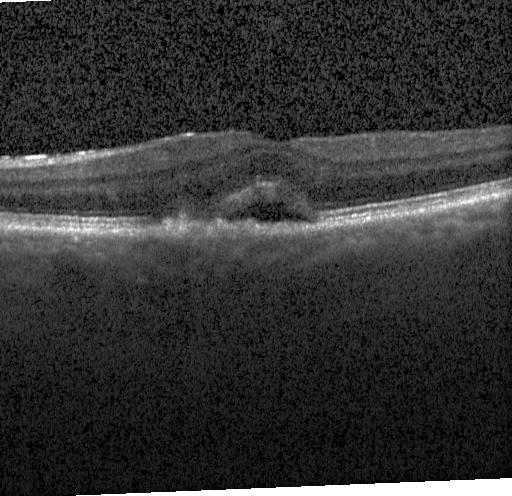 Diagnosis: choroidal neovascularization.